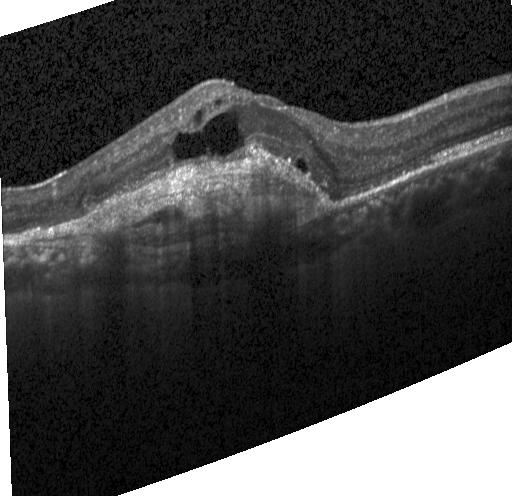
Assessment: choroidal neovascularization.